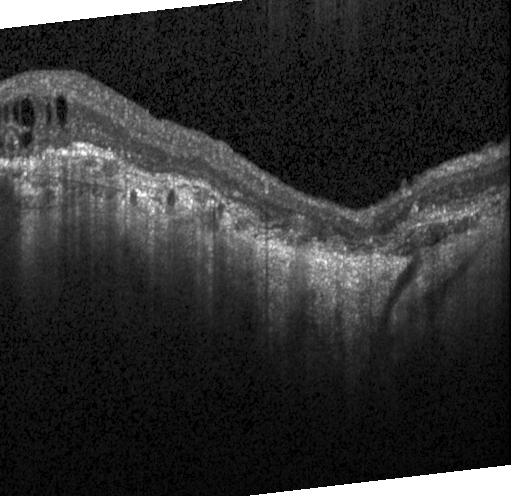

Retinal OCT cross-section
Choroidal neovascularization.